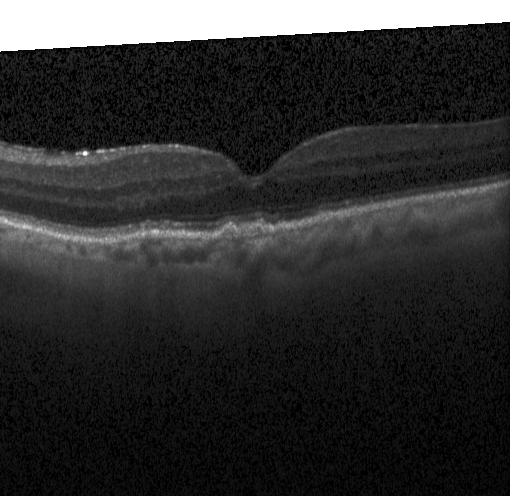 Dx: drusen.